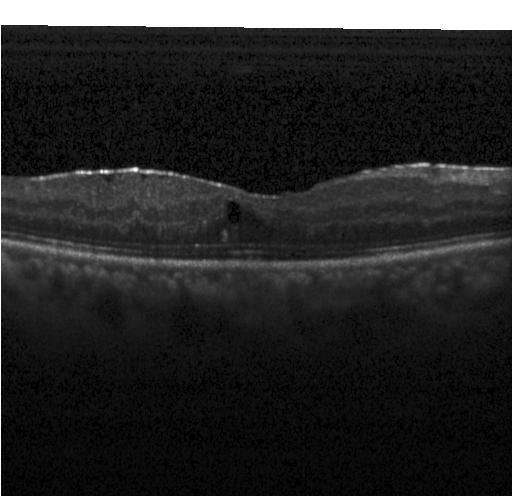

Optical coherence tomography B-scan
Diagnosis: diabetic macular edema (DME).